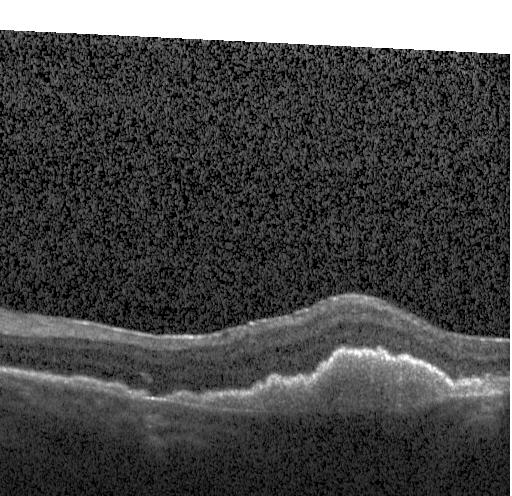
A choroidal neovascular membrane.